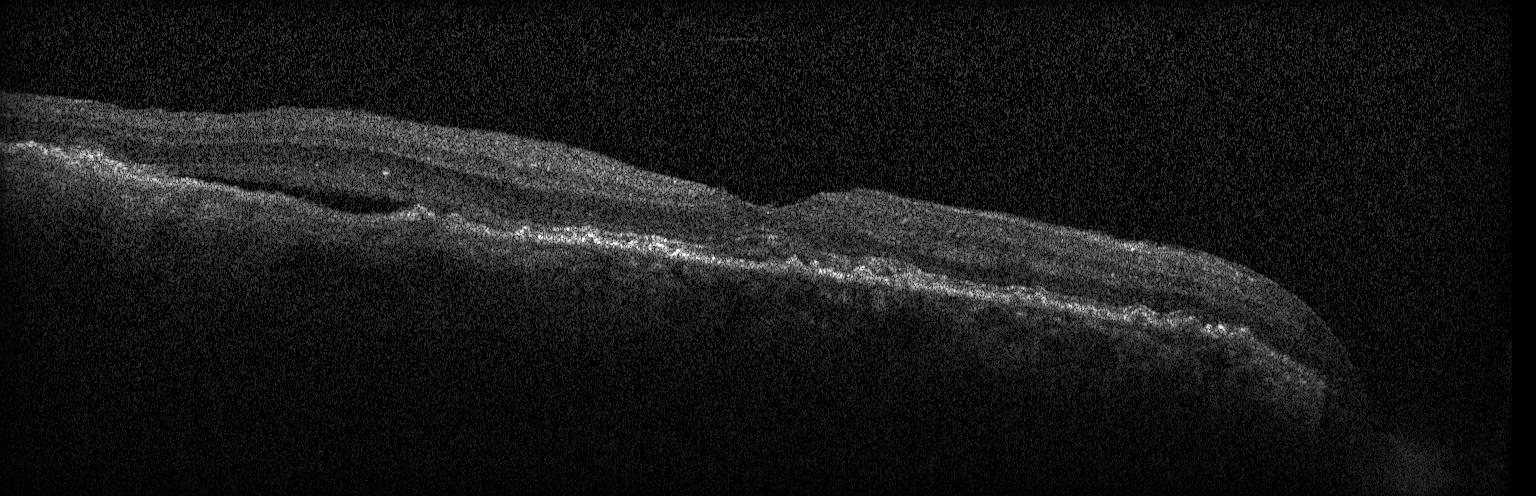

Macular scan. SD-OCT. Optical coherence tomography B-scan. Acquired on a Heidelberg Spectralis.
The scan shows choroidal neovascularization (CNV).